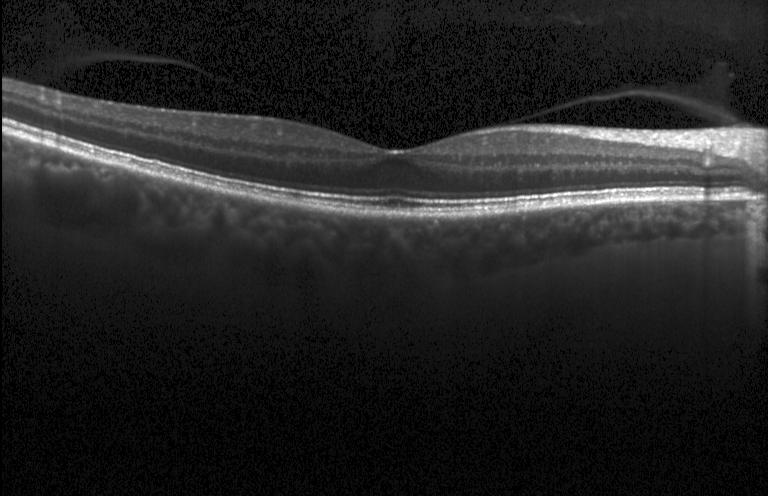
OCT line scan. Diagnosis: neither CNV, DME, nor drusen.